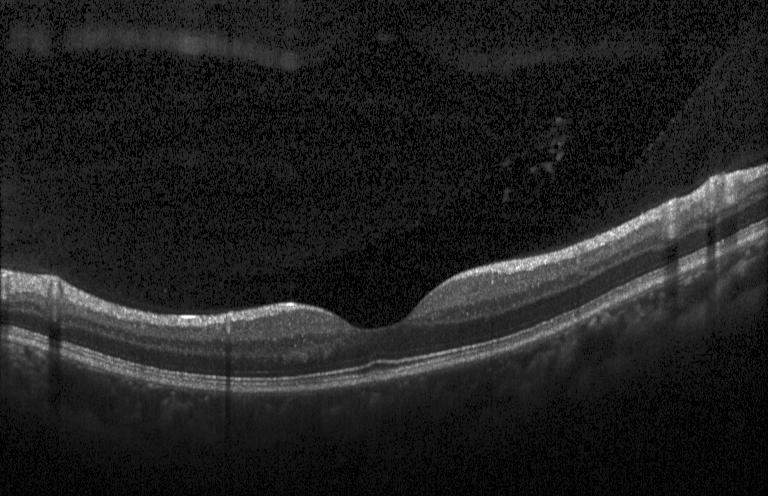 Finding: no choroidal neovascularization, diabetic macular edema, or drusen.